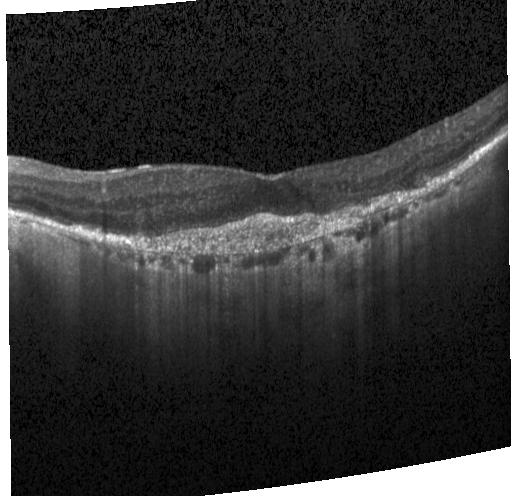 Through the macula, Heidelberg Spectralis OCT system, SD-OCT, OCT B-scan.
Assessment: a choroidal neovascular membrane.